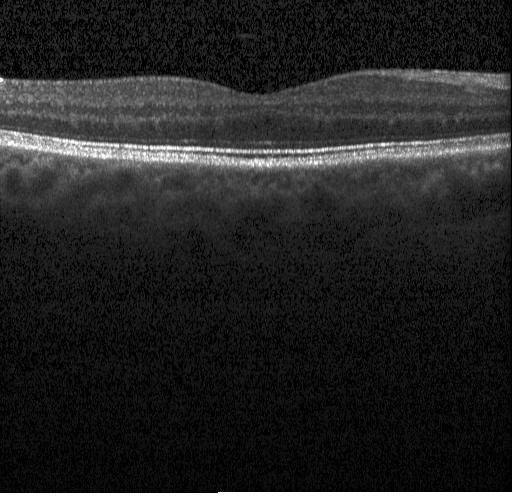 Heidelberg Spectralis OCT system, macular scan, retinal OCT B-scan, spectral-domain OCT — Finding: no choroidal neovascularization, diabetic macular edema, or drusen.